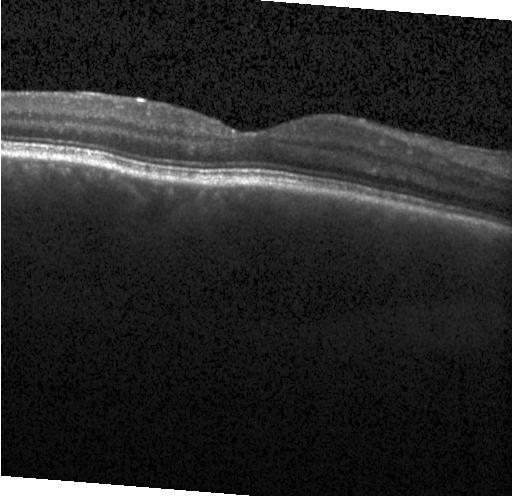

Finding: no choroidal neovascularization, no diabetic macular edema, and no drusen.